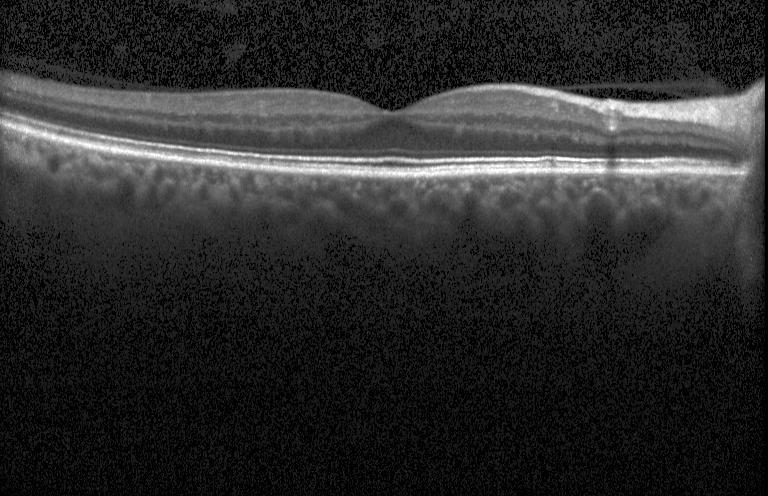

OCT line scan; Heidelberg Spectralis
OCT finding: neither choroidal neovascularization, diabetic macular edema, nor drusen.